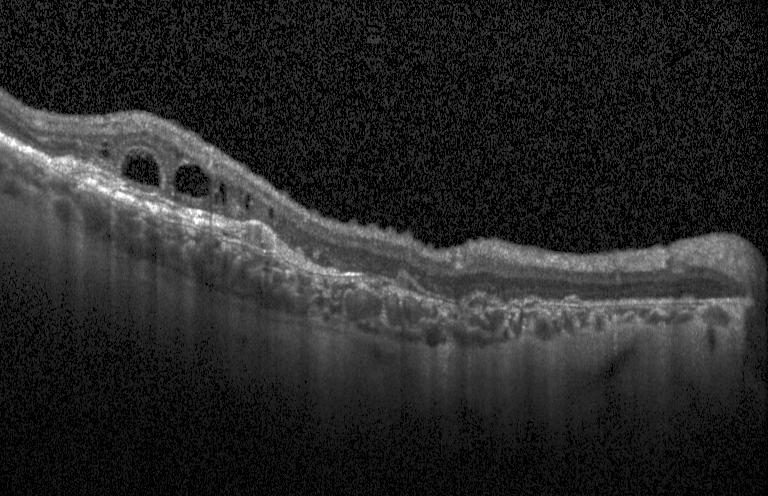 Spectral-domain optical coherence tomography; retinal OCT B-scan; Heidelberg Spectralis OCT system. The scan shows a choroidal neovascular membrane.